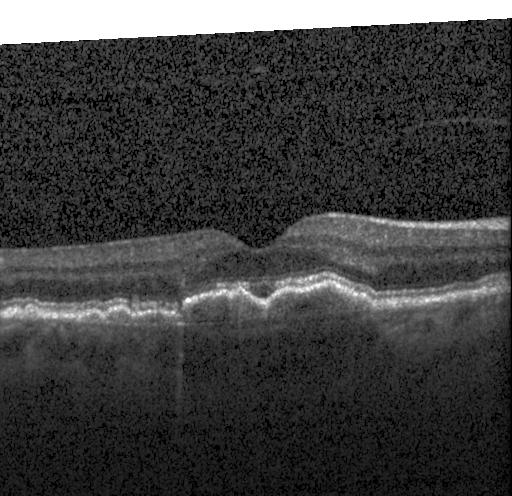 A choroidal neovascular membrane.